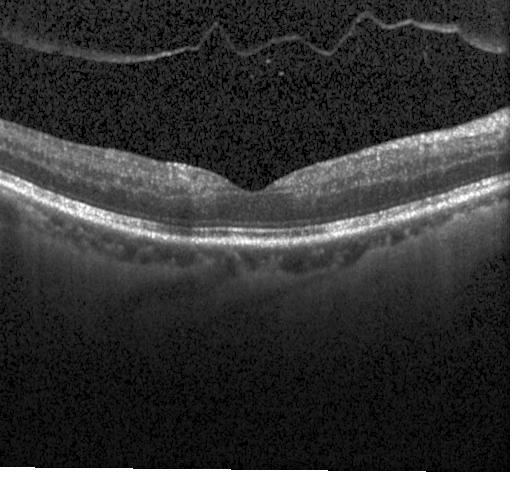
Acquired on a Heidelberg Spectralis; spectral-domain optical coherence tomography; horizontal scan through the fovea; OCT B-scan. Assessment: no choroidal neovascularization, no diabetic macular edema, and no drusen.